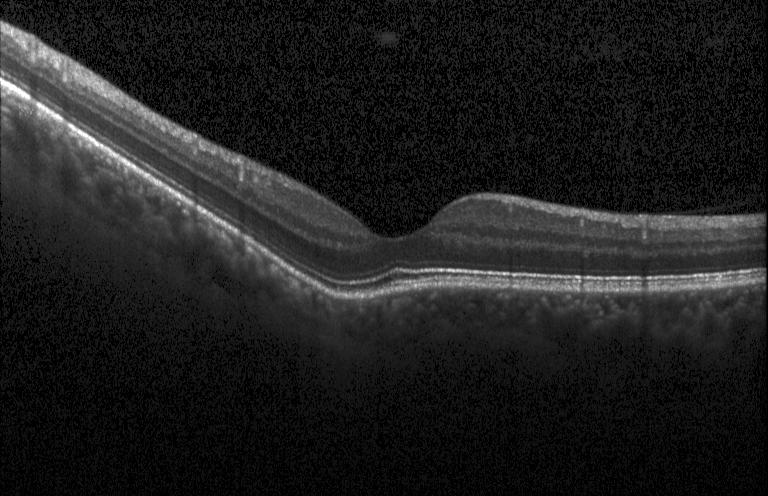 Through the macula; retinal OCT cross-section; Heidelberg Spectralis; spectral-domain optical coherence tomography
Impression: neither choroidal neovascularization, diabetic macular edema, nor drusen.